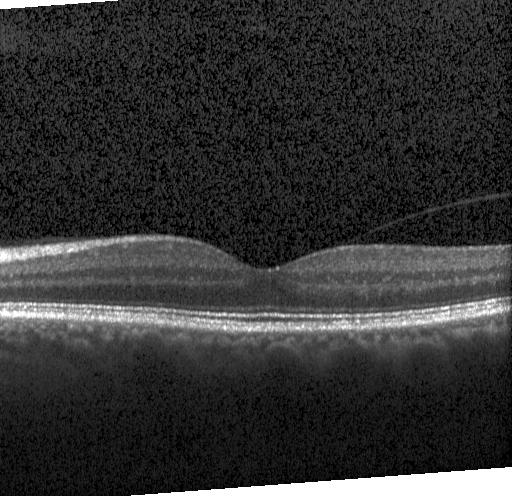 Retinal OCT cross-section.
This B-scan demonstrates no choroidal neovascularization, no diabetic macular edema, and no drusen.